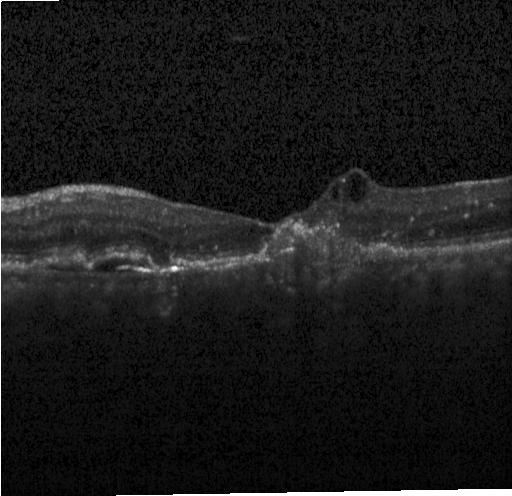

Finding: CNV.